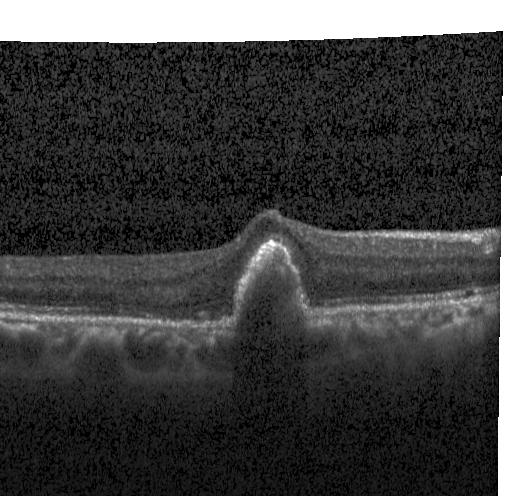

OCT B-scan, spectral-domain OCT. Diagnosis: a choroidal neovascular membrane.